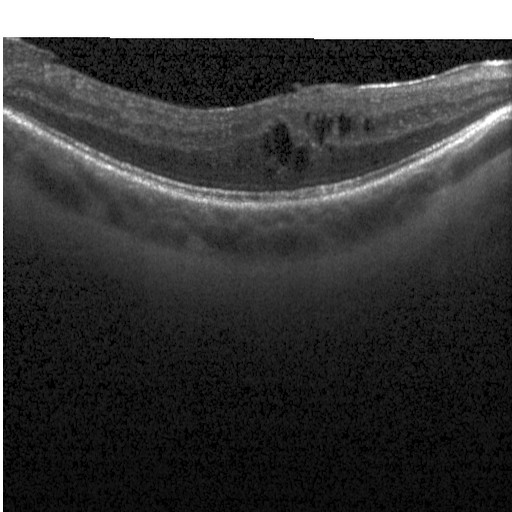
Macular OCT: diabetic macular edema (DME).